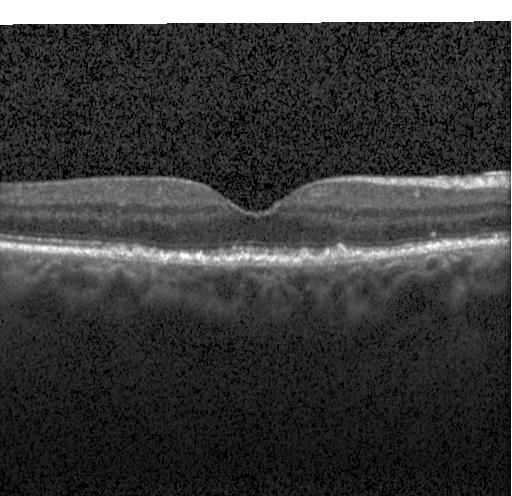 Heidelberg Spectralis, macular scan, OCT line scan, SD-OCT — Impression: drusen.